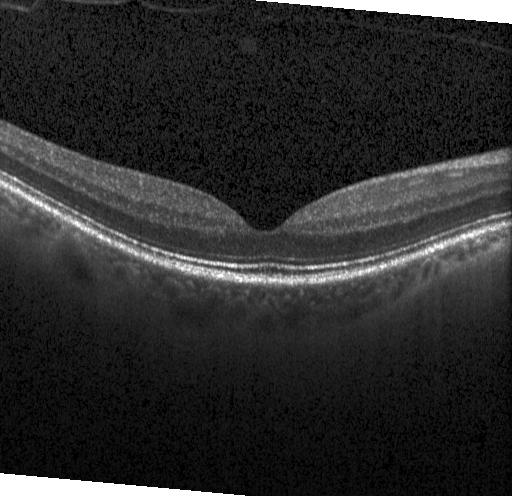 Dx: neither CNV, DME, nor drusen.